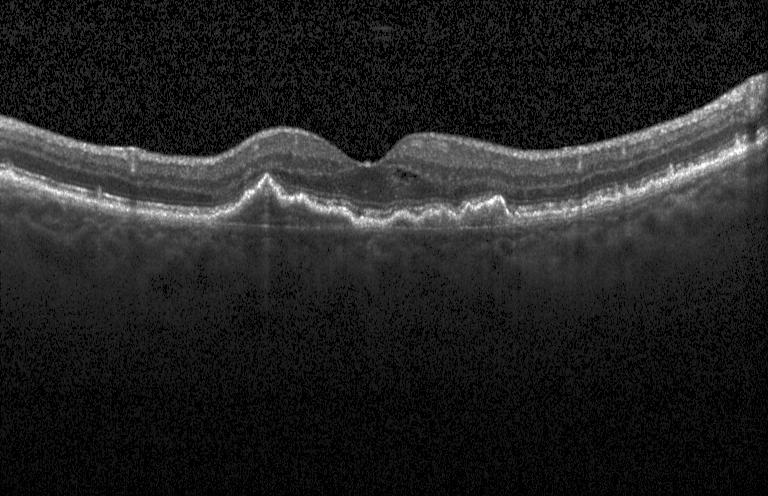 Impression: a choroidal neovascular membrane.